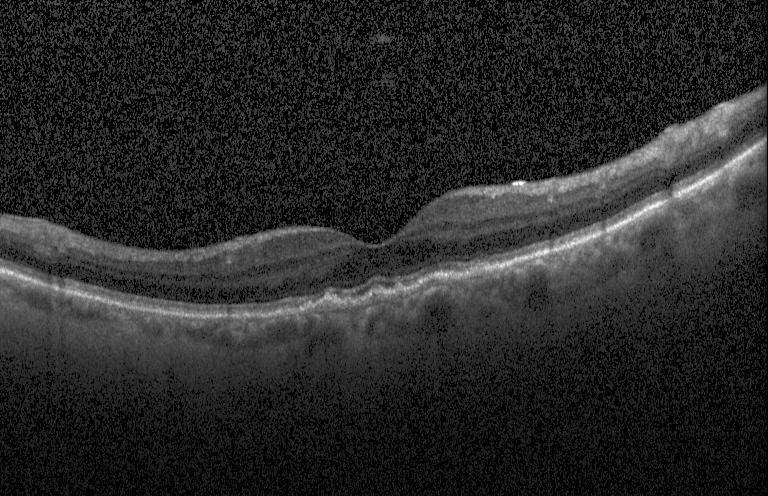

OCT B-scan — Impression: sub-RPE drusenoid deposits.